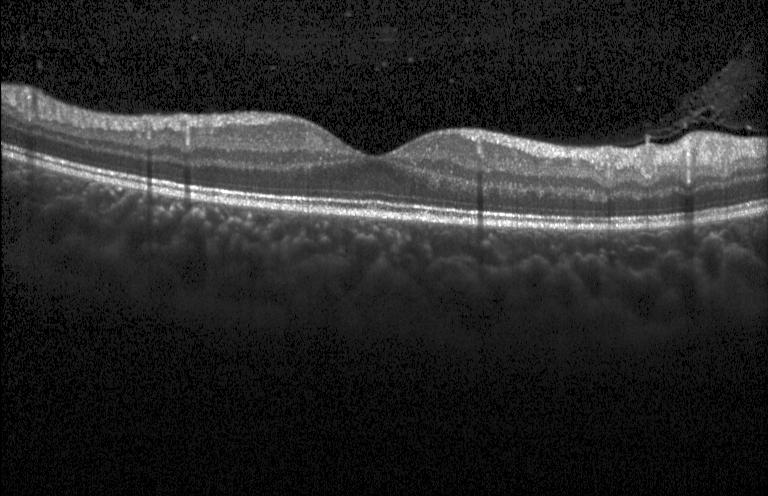 Dx: no CNV, DME, or drusen.